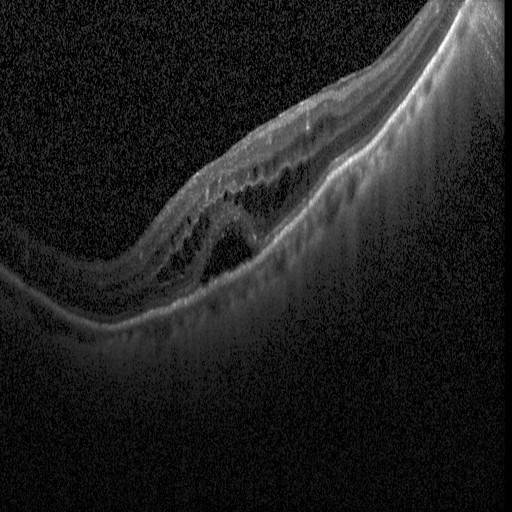
Spectral-domain optical coherence tomography · optical coherence tomography scan · acquired on a Heidelberg Spectralis
Dx: diabetic macular edema (DME).